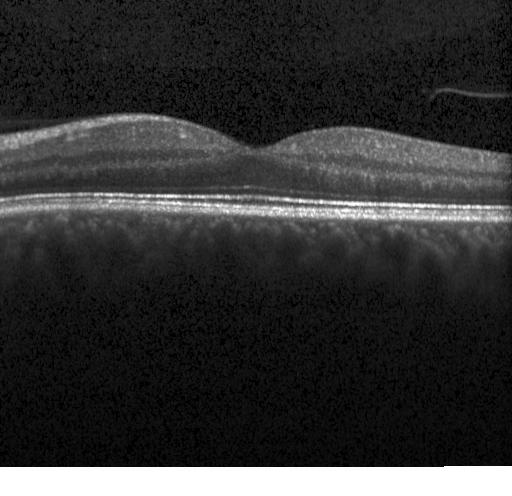
Centered on the fovea; OCT B-scan; instrument: Heidelberg Spectralis. Finding: neither choroidal neovascularization, diabetic macular edema, nor drusen.